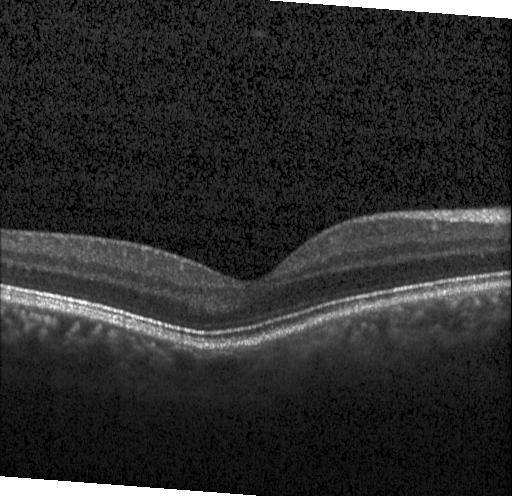

OCT line scan; through the macula.
Impression: neither choroidal neovascularization, diabetic macular edema, nor drusen.